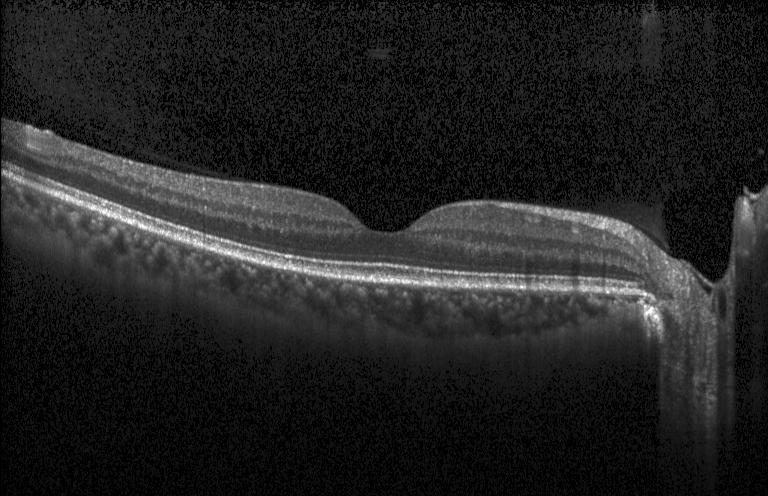 Spectral-domain optical coherence tomography, optical coherence tomography scan. Assessment: no choroidal neovascularization, diabetic macular edema, or drusen.